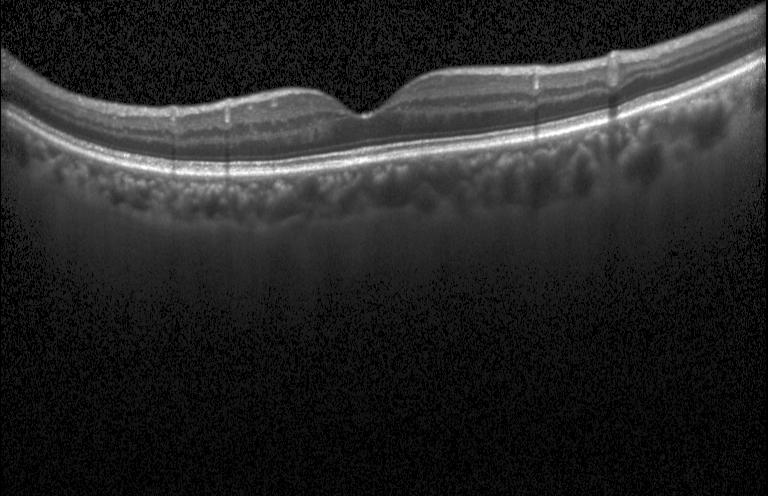
Dx: no choroidal neovascularization, diabetic macular edema, or drusen.